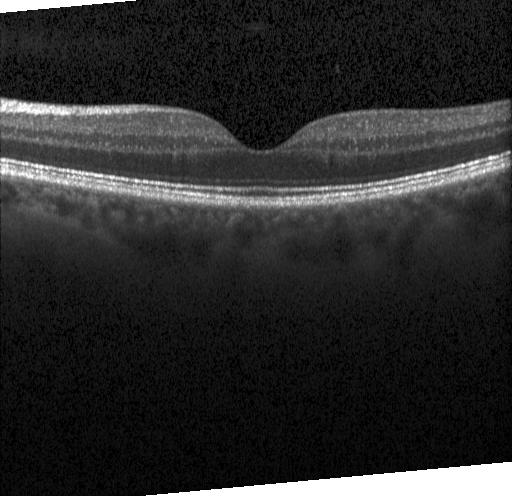 Acquired on a Heidelberg Spectralis. Optical coherence tomography scan.
Impression: neither choroidal neovascularization, diabetic macular edema, nor drusen.